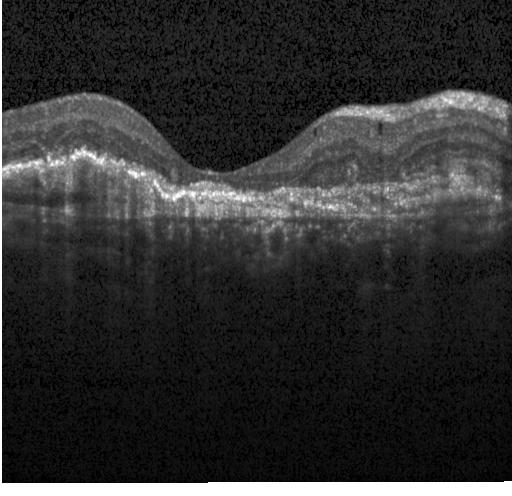

Retinal OCT B-scan. Spectral-domain optical coherence tomography — Finding: a choroidal neovascular membrane.